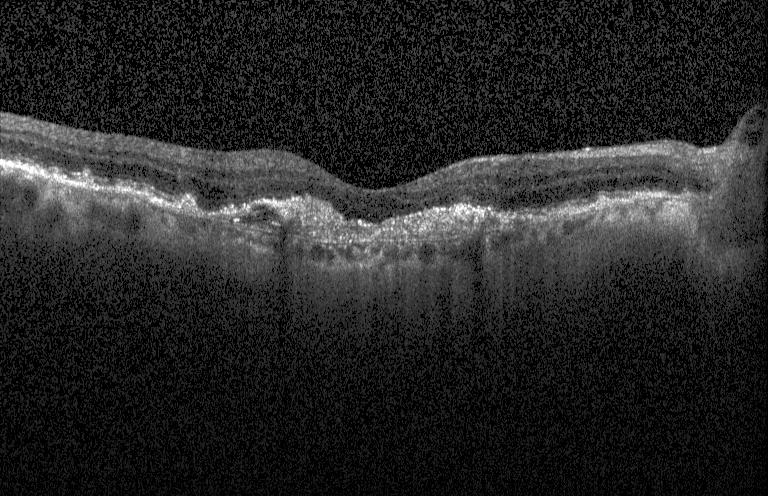

Impression: a choroidal neovascular membrane.